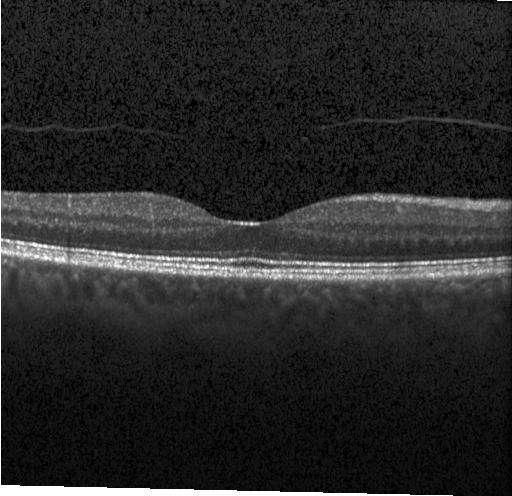

Assessment: no choroidal neovascularization, no diabetic macular edema, and no drusen.